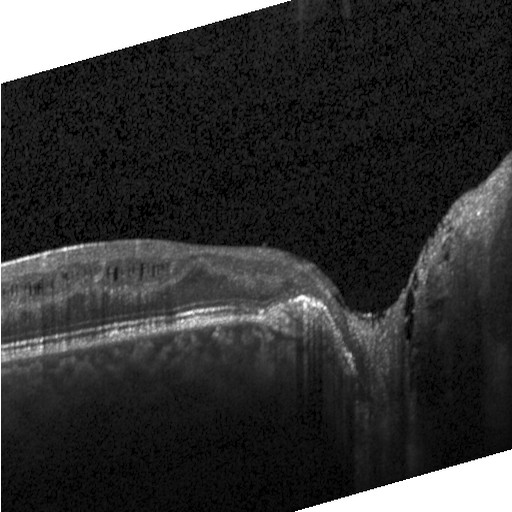 Macular OCT: diabetic macular edema.